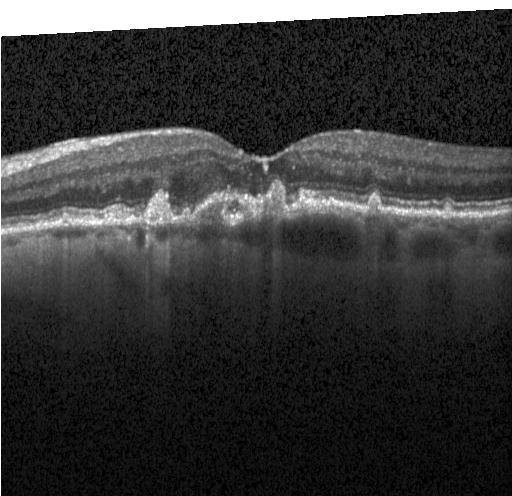

Retinal OCT cross-section; through the macula — Macular OCT: a choroidal neovascular membrane.